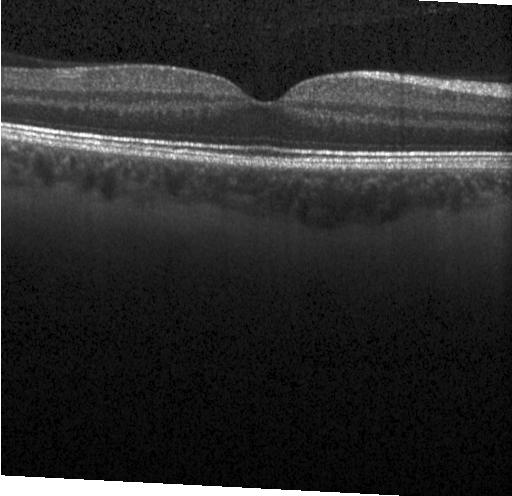 Dx: no choroidal neovascularization, no diabetic macular edema, and no drusen.